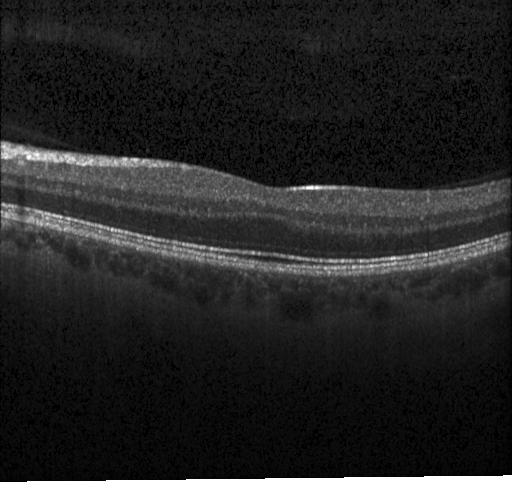

Spectral-domain OCT B-scan: neither choroidal neovascularization, diabetic macular edema, nor drusen.